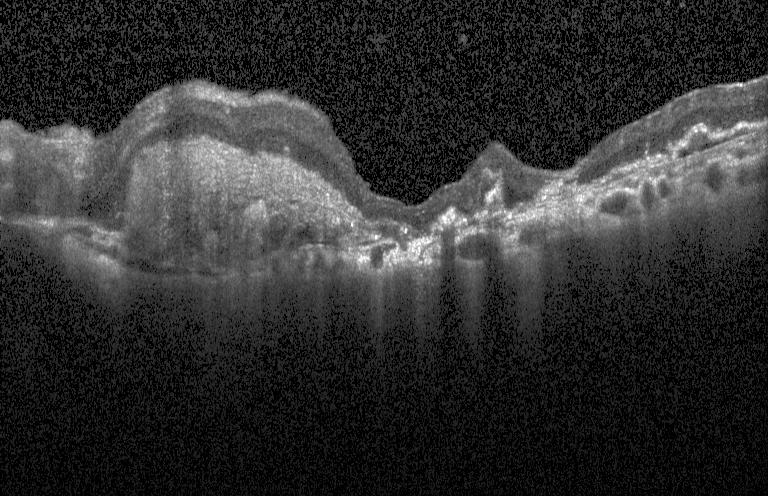
Through the macula, instrument: Heidelberg Spectralis, retinal OCT B-scan, SD-OCT.
This B-scan demonstrates a choroidal neovascular membrane.